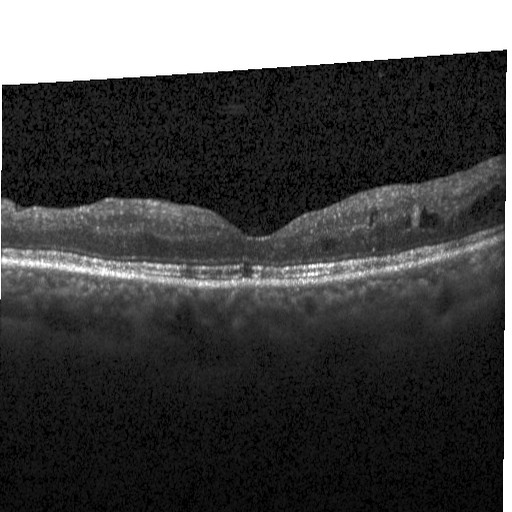
Horizontal scan through the fovea. Heidelberg Spectralis. OCT line scan
The scan shows DME.